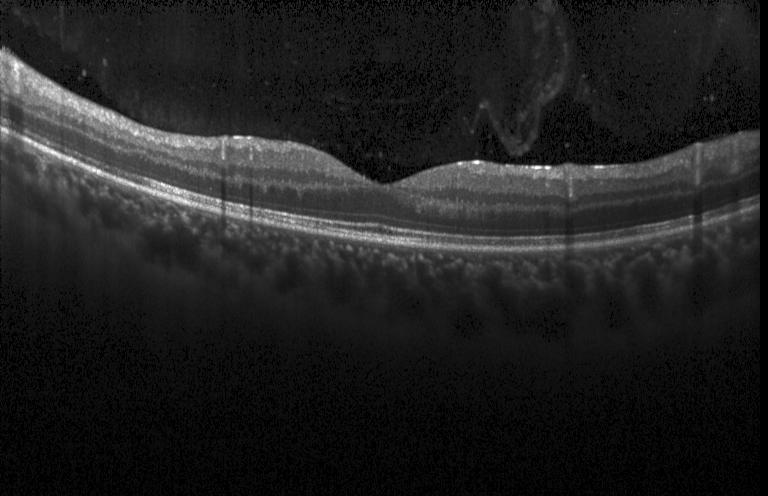
Macular scan. OCT B-scan — Diagnosis: neither choroidal neovascularization, diabetic macular edema, nor drusen.